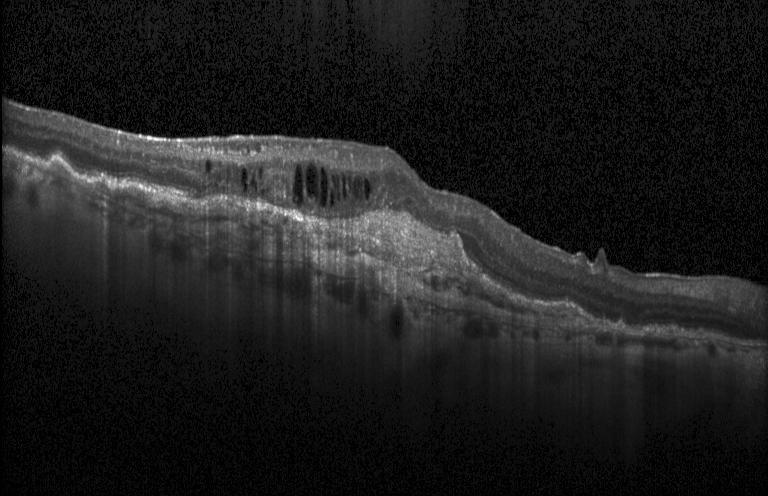 Retinal OCT B-scan — The scan shows a choroidal neovascular membrane.